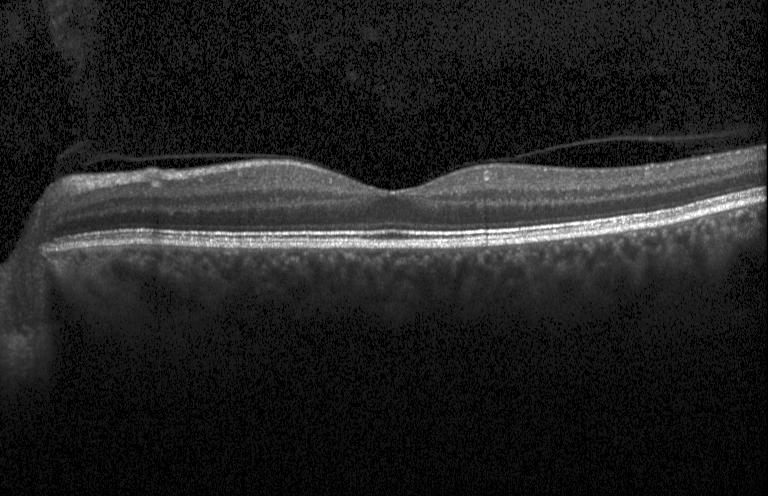
Diagnosis: no CNV, DME, or drusen.